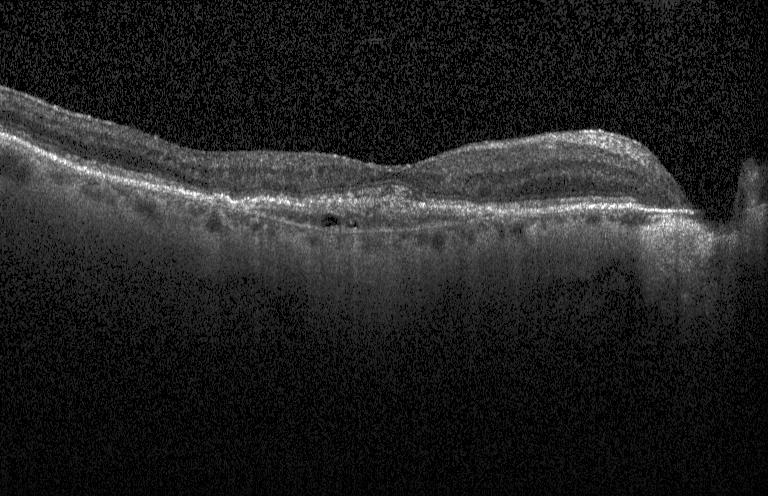
A choroidal neovascular membrane.